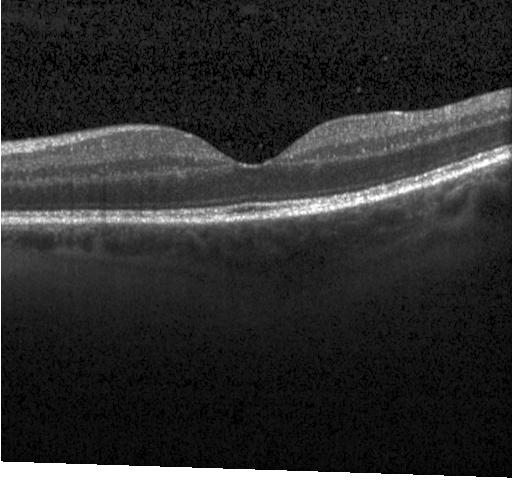
This B-scan demonstrates no choroidal neovascularization, diabetic macular edema, or drusen.